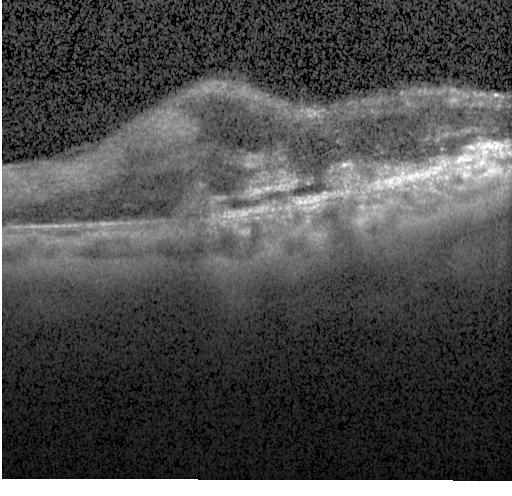

Assessment: a choroidal neovascular membrane.